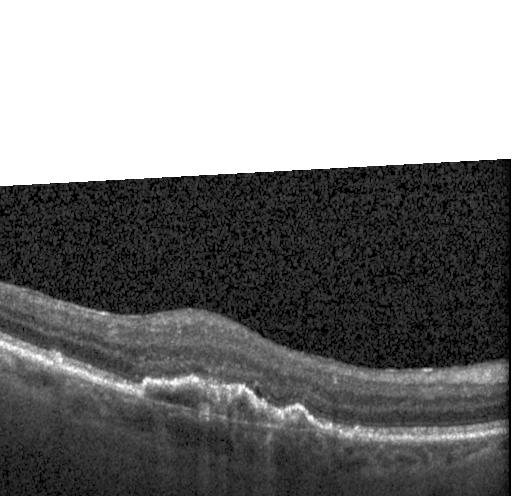 OCT scan showing choroidal neovascularization.